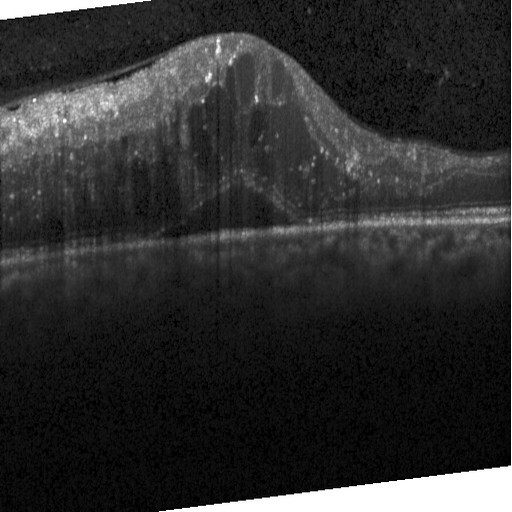

Finding: diabetic macular edema.